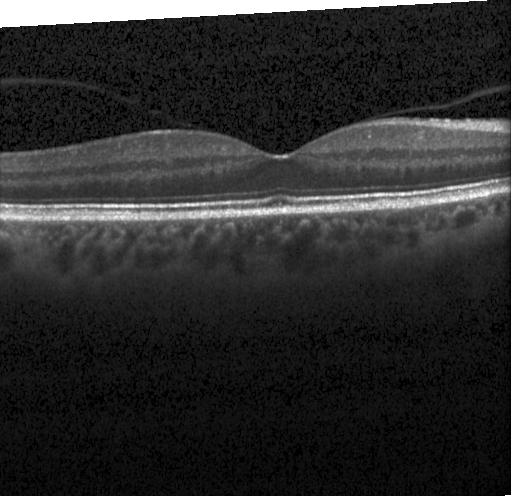

Heidelberg Spectralis; optical coherence tomography B-scan — Macular OCT: no evidence of choroidal neovascularization, diabetic macular edema, or drusen.